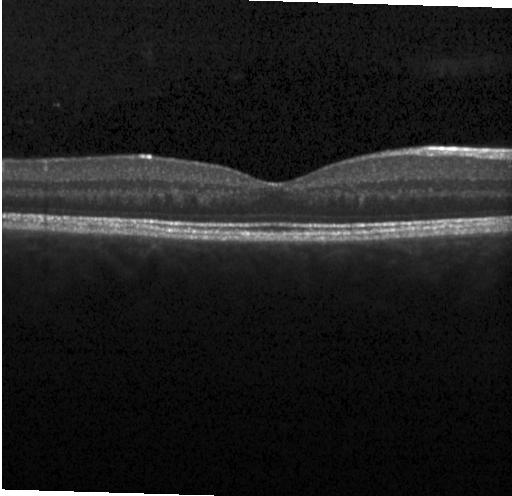

Horizontal scan through the fovea · OCT B-scan. Diagnosis: no choroidal neovascularization, no diabetic macular edema, and no drusen.